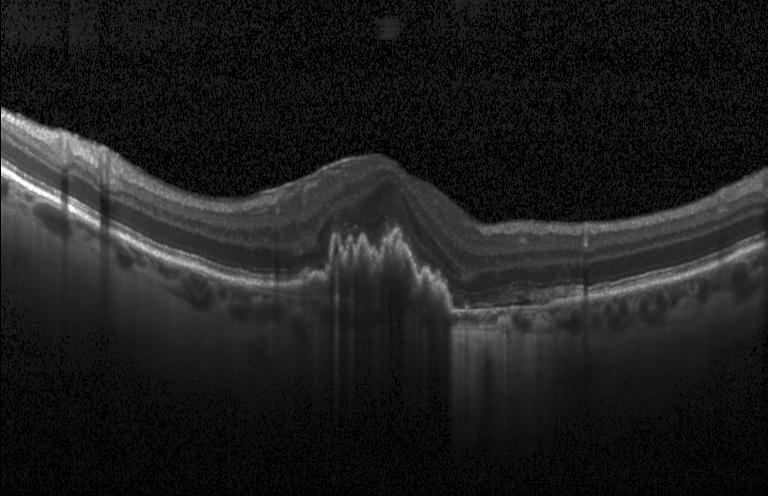 Assessment: a choroidal neovascular membrane.